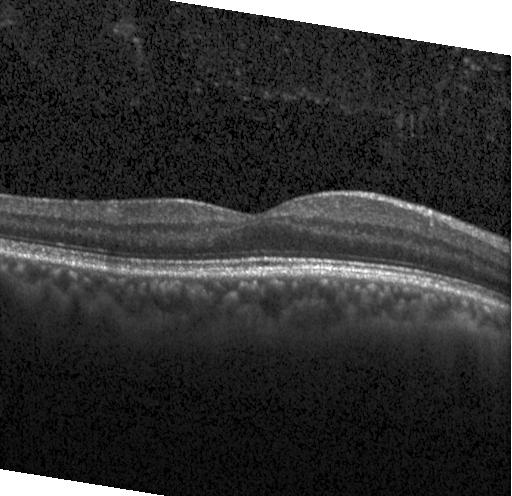
Horizontal scan through the fovea; optical coherence tomography scan; instrument: Heidelberg Spectralis. Diagnosis: neither CNV, DME, nor drusen.